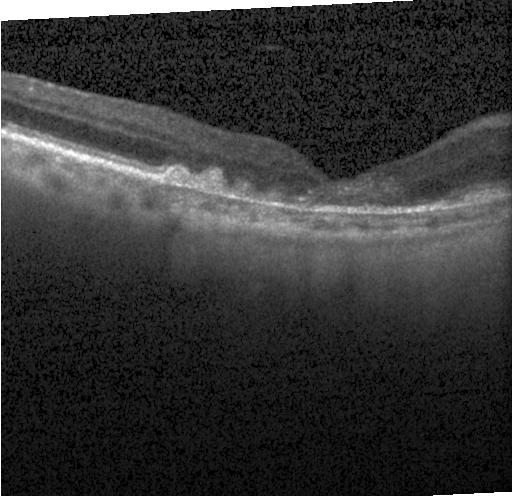

This B-scan demonstrates a choroidal neovascular membrane.